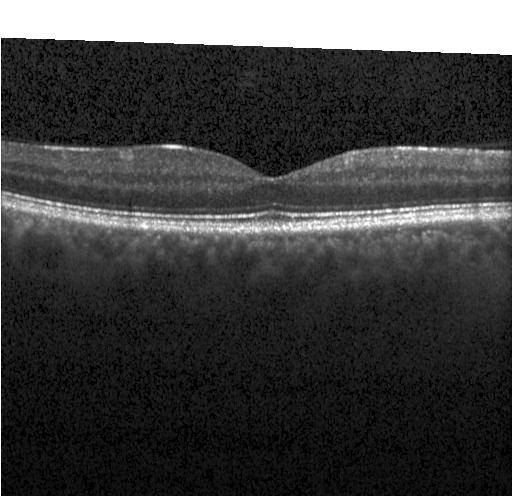 Diagnosis: no CNV, no DME, and no drusen.